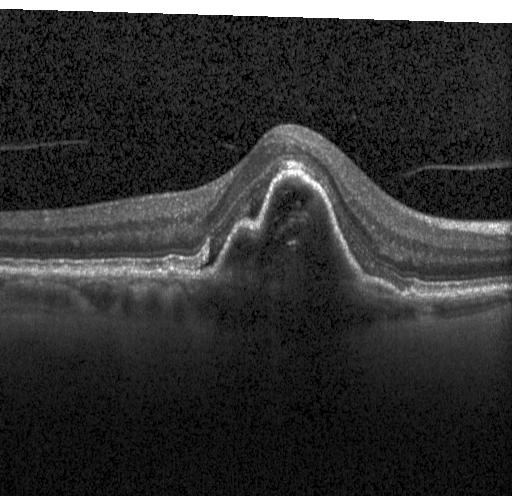
Macular OCT demonstrating CNV.